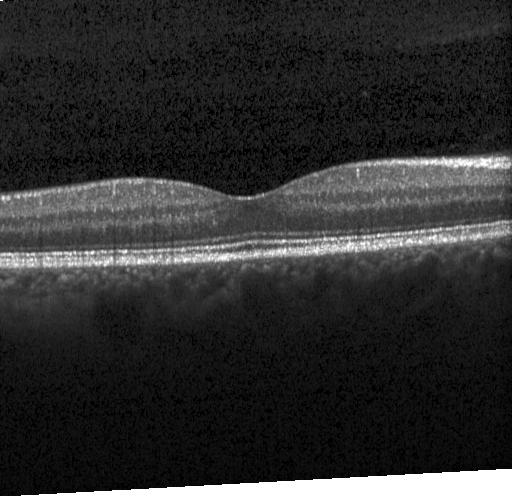

OCT line scan; through the macula; spectral-domain OCT; acquired on a Heidelberg Spectralis.
This B-scan demonstrates no choroidal neovascularization, diabetic macular edema, or drusen.